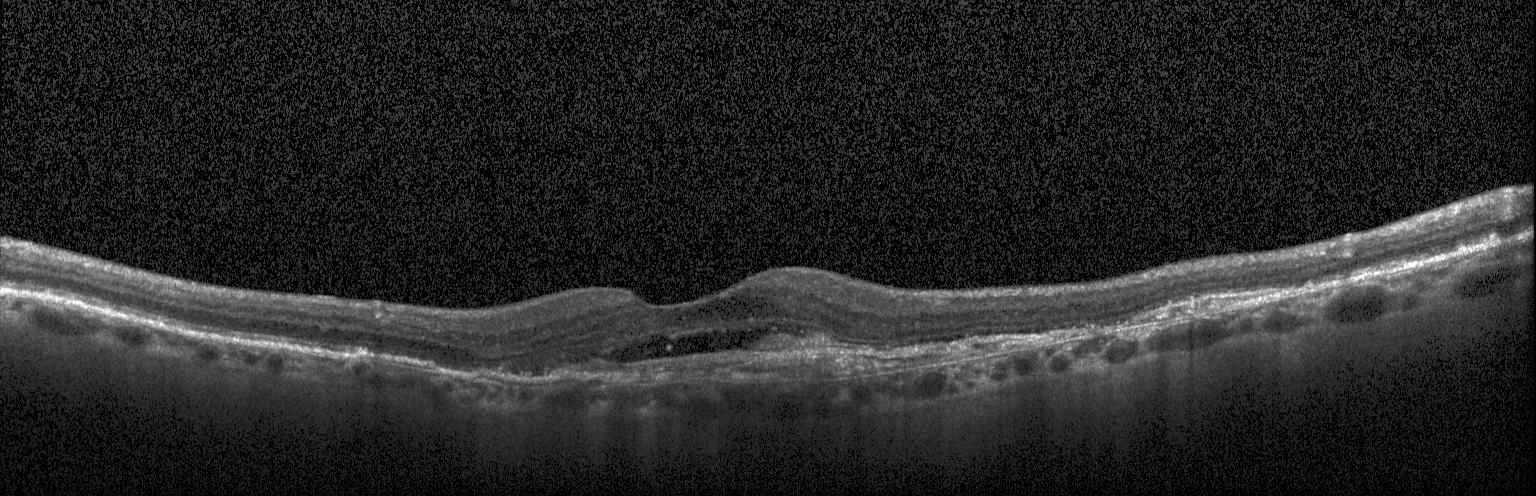

Horizontal scan through the fovea · spectral-domain OCT · Heidelberg Spectralis OCT system · optical coherence tomography B-scan.
Impression: a choroidal neovascular membrane.